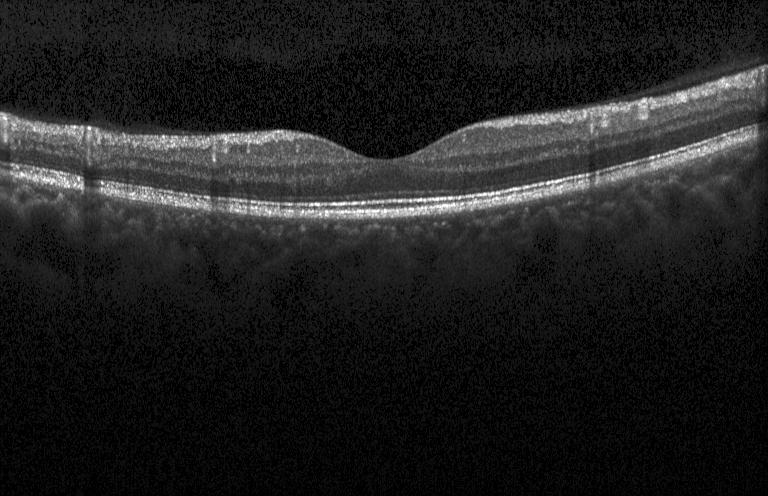
OCT line scan. Spectral-domain optical coherence tomography. Macular scan — Assessment: neither CNV, DME, nor drusen.